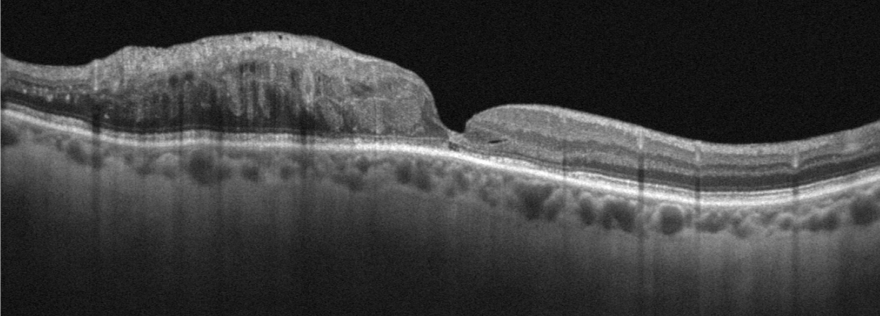
Macular scan, optical coherence tomography scan, Optovue Avanti RTVue XR
This B-scan demonstrates diabetic macular edema (DME).